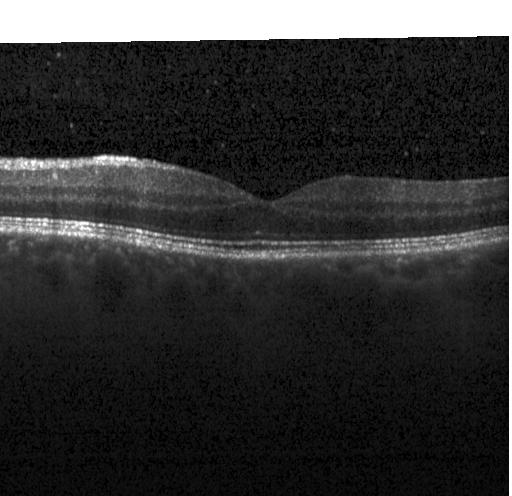
Acquired on a Heidelberg Spectralis, spectral-domain OCT, OCT B-scan, through the macula.
Assessment: no evidence of choroidal neovascularization, diabetic macular edema, or drusen.